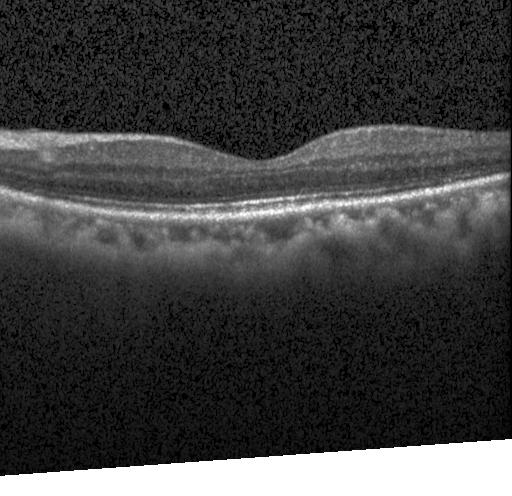

Macular scan, SD-OCT, acquired on a Heidelberg Spectralis, OCT line scan.
Finding: neither choroidal neovascularization, diabetic macular edema, nor drusen.